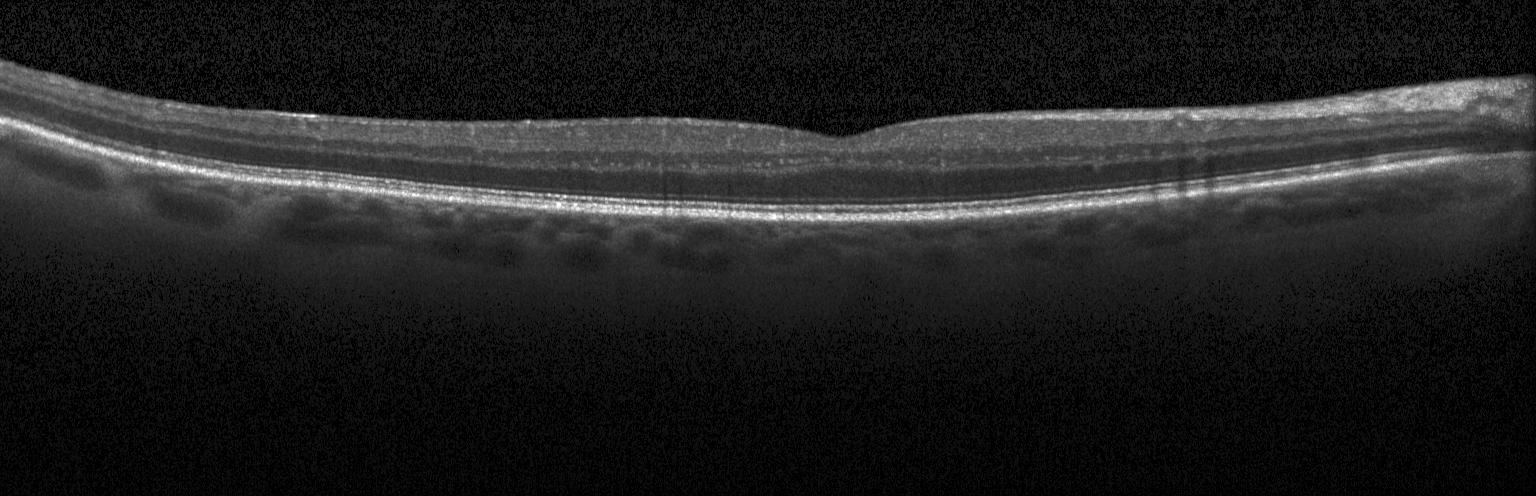
Diagnosis: no CNV, no DME, and no drusen.